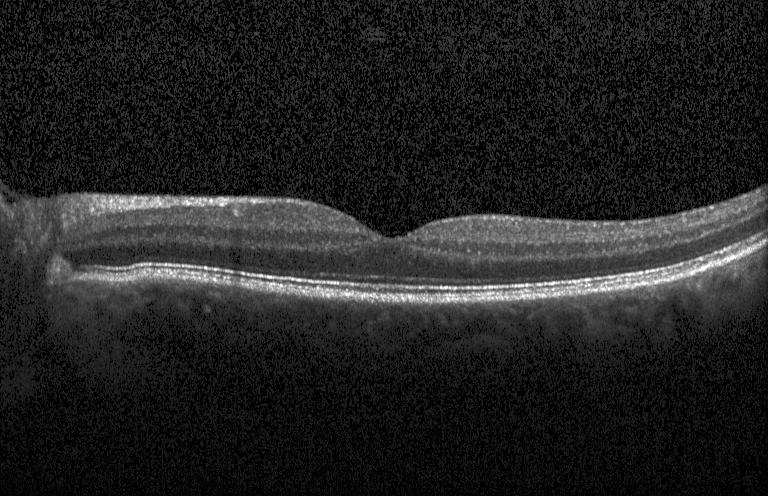
Dx: no choroidal neovascularization, no diabetic macular edema, and no drusen.